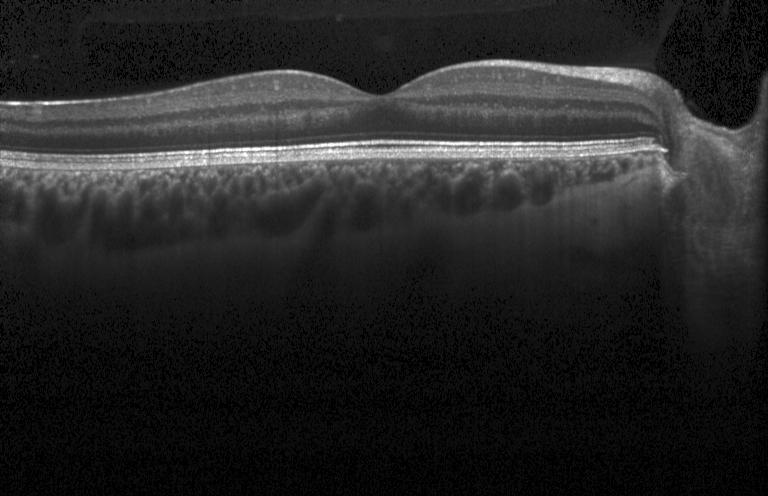
Retinal OCT B-scan. This B-scan demonstrates no evidence of CNV, DME, or drusen.